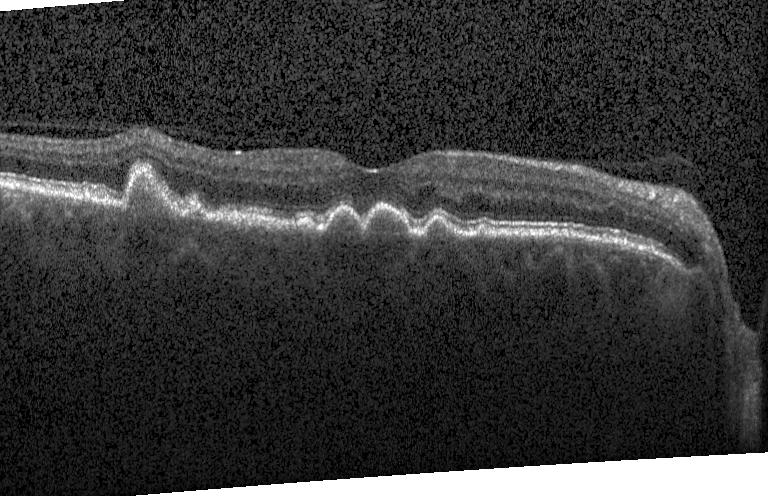

Macular OCT: drusen.